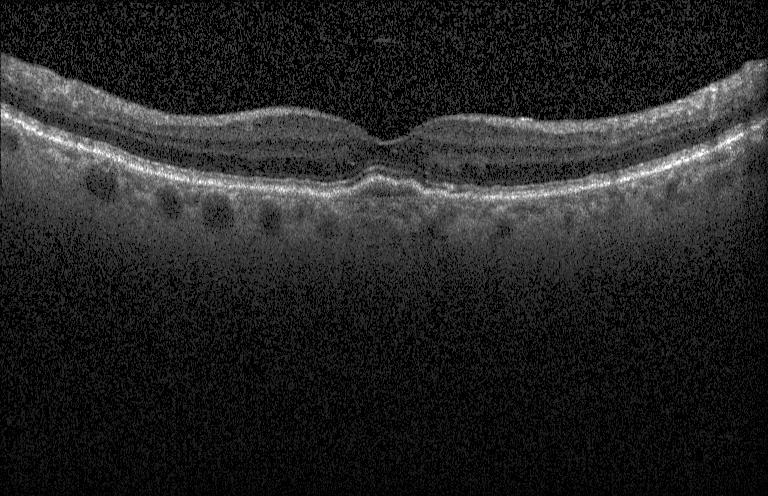

Optical coherence tomography scan; fovea-centered.
Finding: a choroidal neovascular membrane.